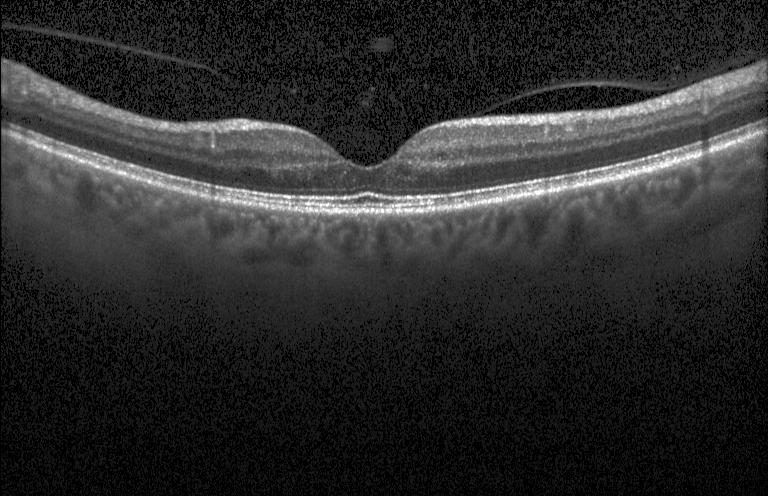 Spectral-domain OCT; optical coherence tomography B-scan — Macular OCT: no CNV, no DME, and no drusen.